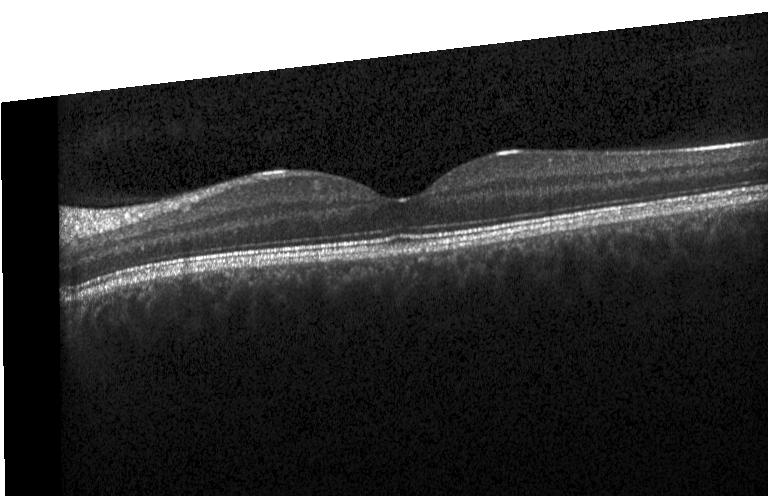
OCT B-scan. Horizontal scan through the fovea. Heidelberg Spectralis — Macular OCT: no evidence of choroidal neovascularization, diabetic macular edema, or drusen.